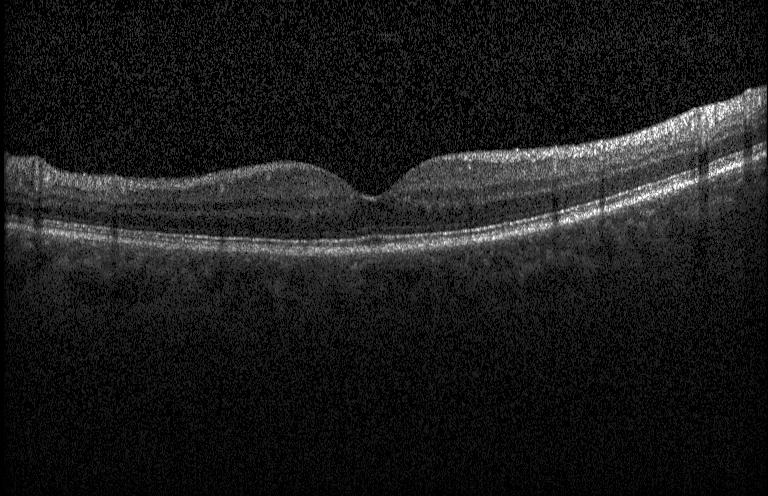 Acquired on a Heidelberg Spectralis · OCT B-scan
Impression: no CNV, no DME, and no drusen.